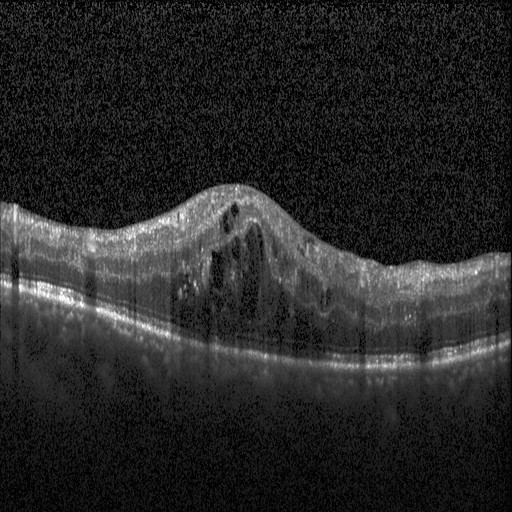

Macular OCT demonstrating diabetic macular edema (DME).